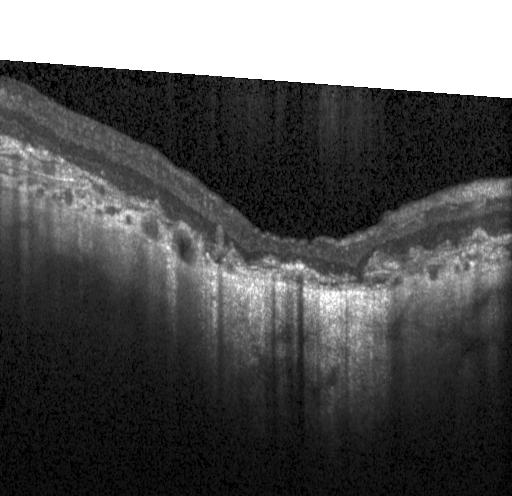

Assessment: a choroidal neovascular membrane.